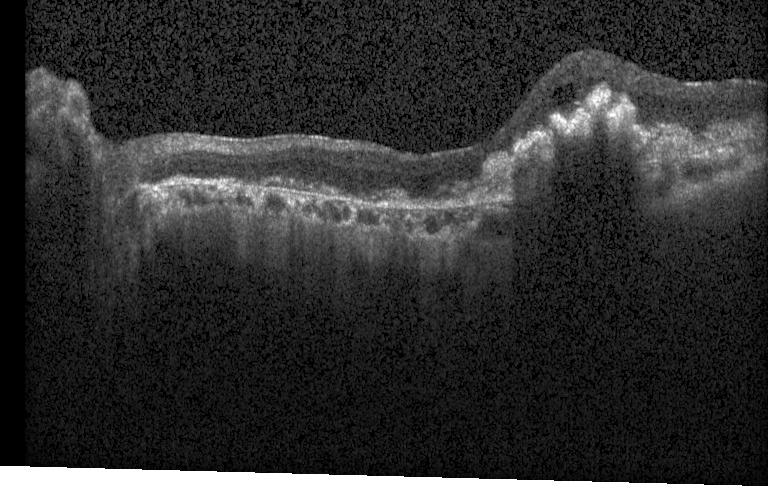

OCT finding: choroidal neovascularization.